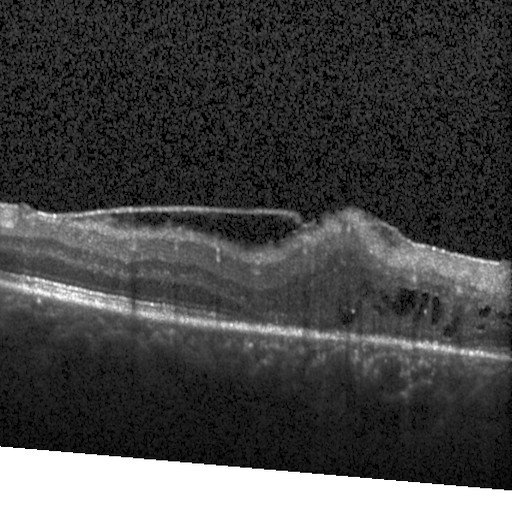
Retinal OCT cross-section.
OCT finding: diabetic macular edema.